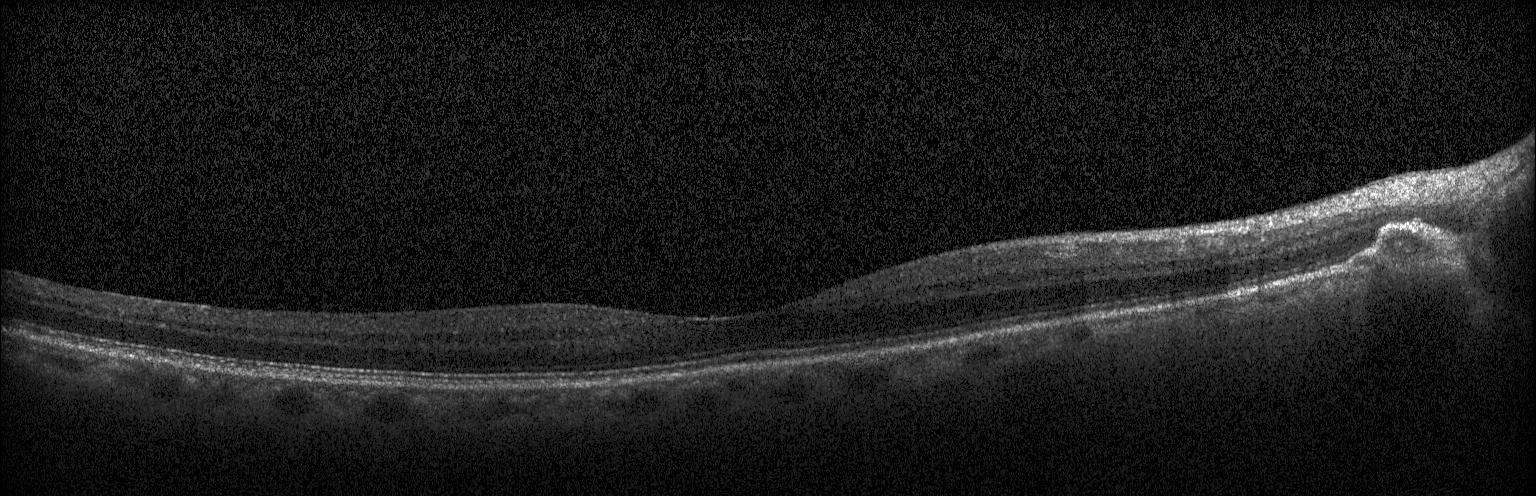 Impression: a choroidal neovascular membrane.